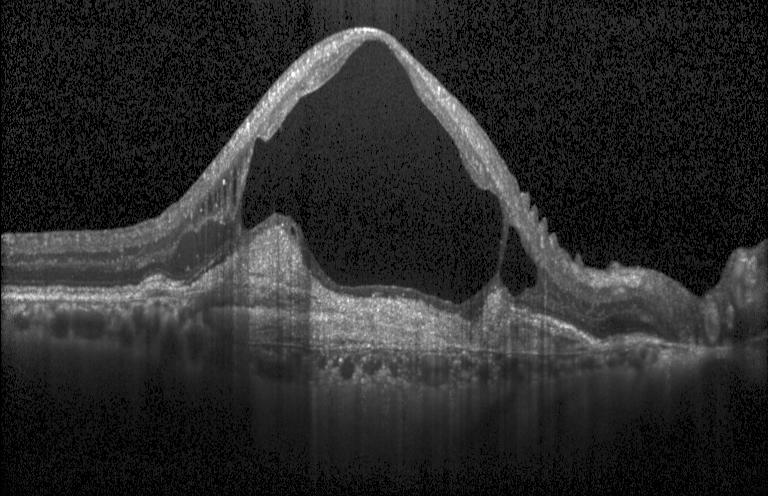 Macular OCT: a choroidal neovascular membrane.